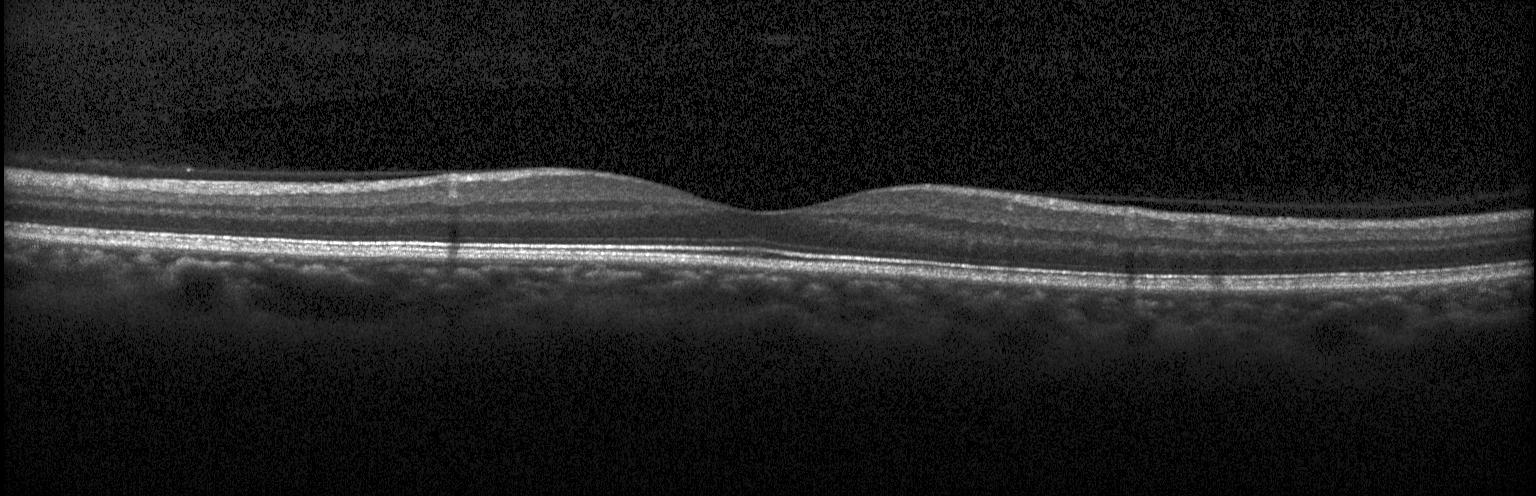 Spectral-domain OCT. Retinal OCT B-scan. Heidelberg Spectralis OCT system. Fovea-centered.
The scan shows neither CNV, DME, nor drusen.